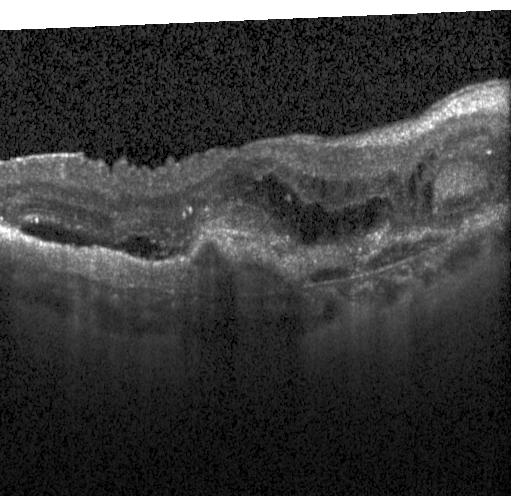

Spectral-domain optical coherence tomography; fovea-centered; Heidelberg Spectralis; optical coherence tomography B-scan — Impression: choroidal neovascularization.